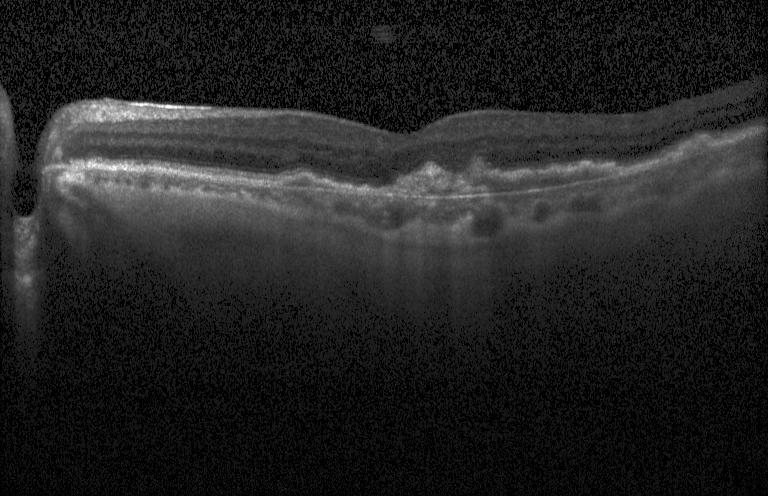

Retinal OCT B-scan. SD-OCT. Macular scan. Heidelberg Spectralis OCT system. Impression: a choroidal neovascular membrane.